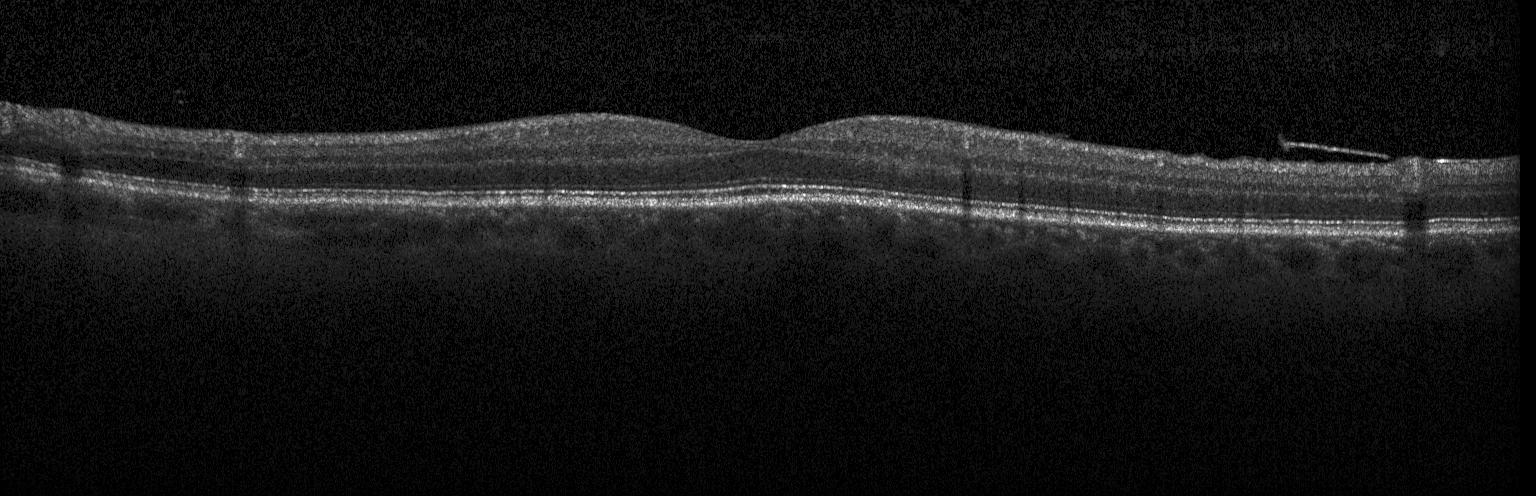 OCT line scan, through the macula, Heidelberg Spectralis OCT system
Impression: no choroidal neovascularization, no diabetic macular edema, and no drusen.